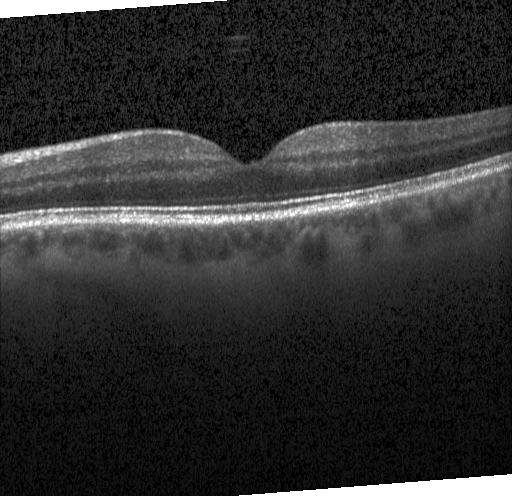

Assessment: neither choroidal neovascularization, diabetic macular edema, nor drusen.